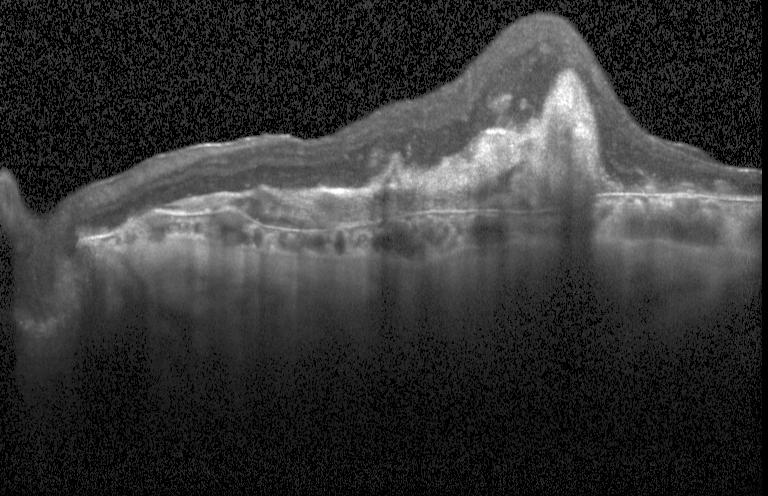 Finding: a choroidal neovascular membrane.